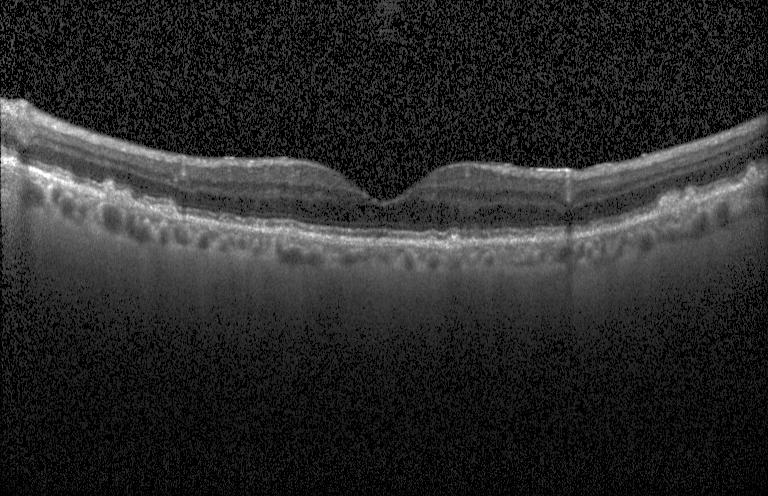
OCT line scan, spectral-domain OCT, through the macula.
Diagnosis: sub-RPE drusenoid deposits.